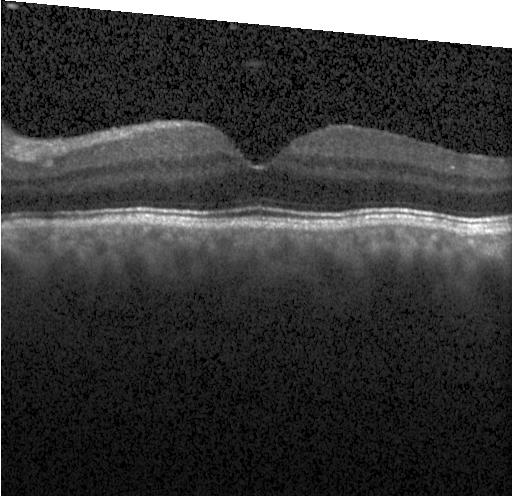

Optical coherence tomography scan — Dx: neither CNV, DME, nor drusen.